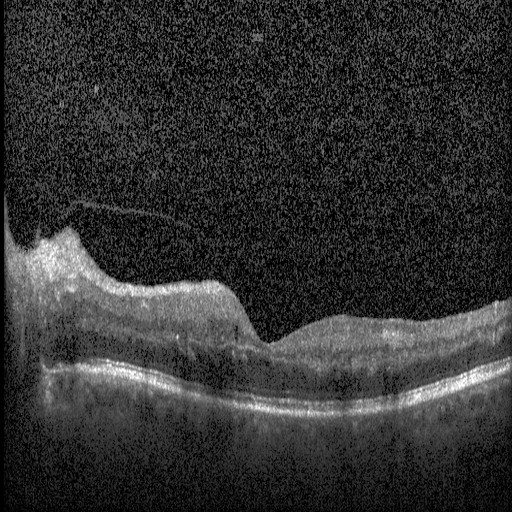 Fovea-centered · optical coherence tomography B-scan · Heidelberg Spectralis — Finding: DME.